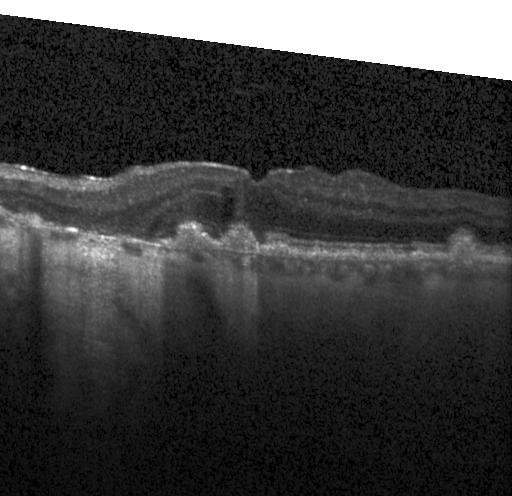

Fovea-centered, Heidelberg Spectralis, retinal OCT B-scan, spectral-domain OCT
Finding: choroidal neovascularization.